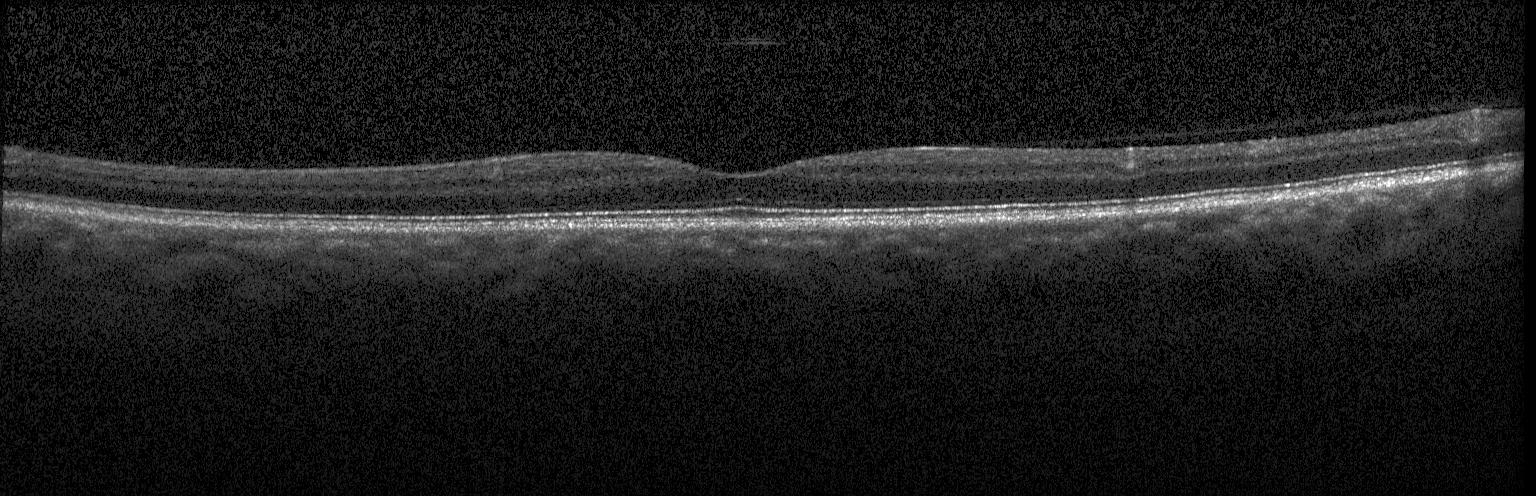

Spectral-domain OCT · OCT line scan · macular scan. Assessment: neither choroidal neovascularization, diabetic macular edema, nor drusen.